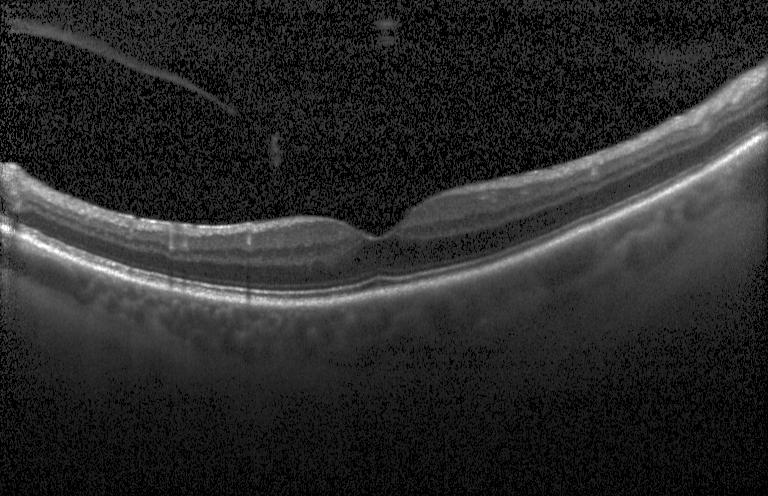
Optical coherence tomography B-scan
Dx: neither CNV, DME, nor drusen.